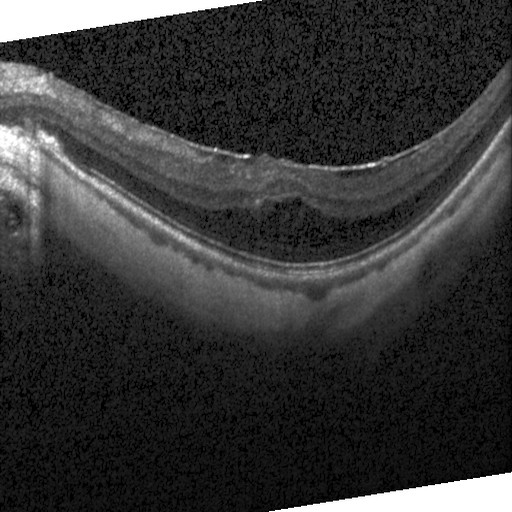

Optical coherence tomography B-scan · instrument: Heidelberg Spectralis · spectral-domain OCT
Finding: DME.